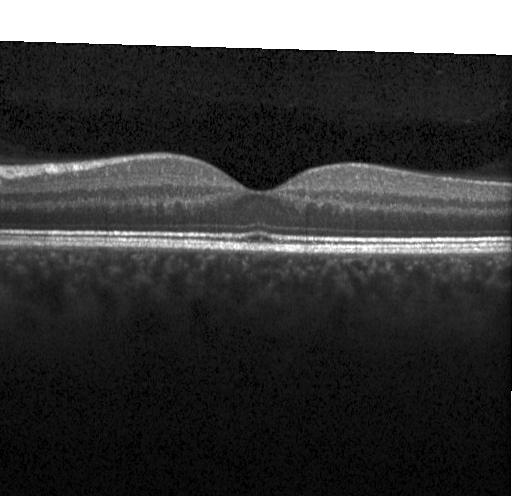 Instrument: Heidelberg Spectralis. Centered on the fovea. SD-OCT. Optical coherence tomography B-scan — This B-scan demonstrates no evidence of choroidal neovascularization, diabetic macular edema, or drusen.